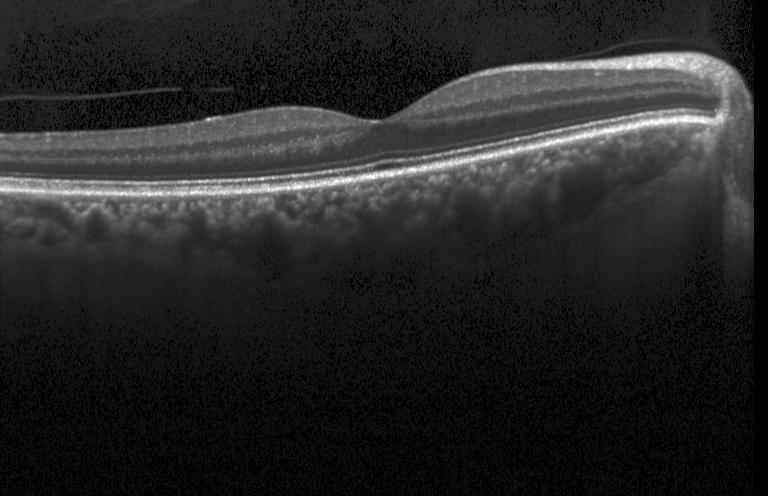 Retinal OCT B-scan; spectral-domain optical coherence tomography; acquired on a Heidelberg Spectralis; through the macula — Impression: no choroidal neovascularization, no diabetic macular edema, and no drusen.